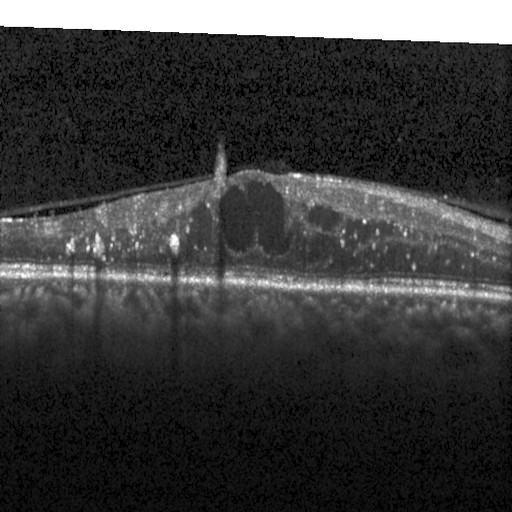
OCT line scan — Diagnosis: diabetic macular edema (DME).